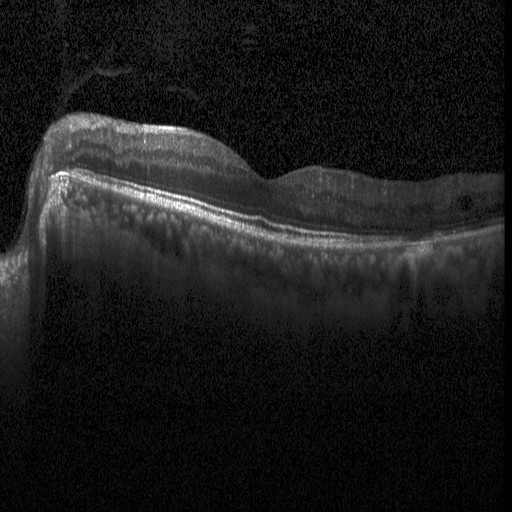

OCT line scan. SD-OCT.
Dx: diabetic macular edema (DME).